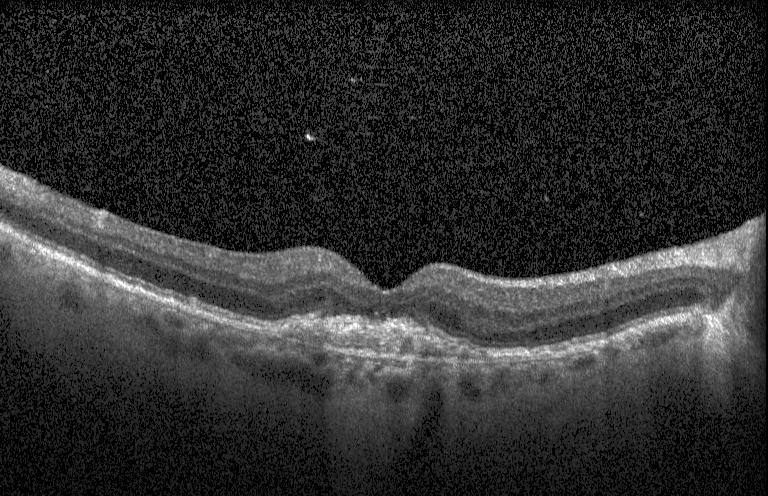 Optical coherence tomography scan · spectral-domain OCT · fovea-centered · Heidelberg Spectralis — The scan shows choroidal neovascularization.